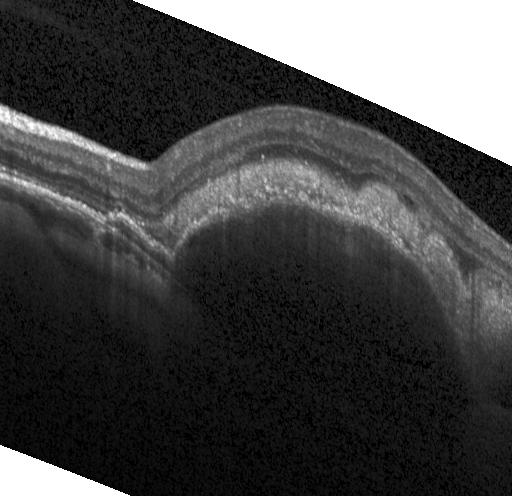 Diagnosis: a choroidal neovascular membrane.